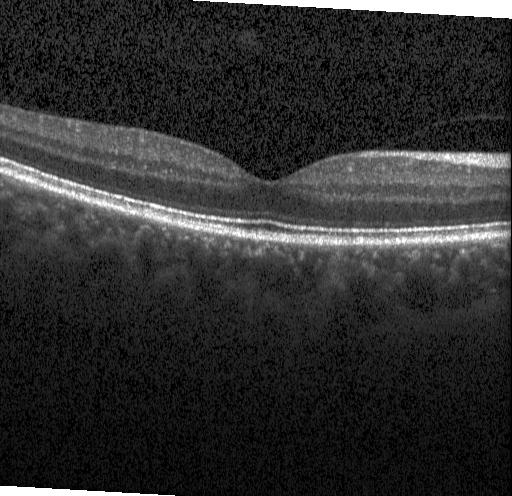 Impression: no evidence of choroidal neovascularization, diabetic macular edema, or drusen.